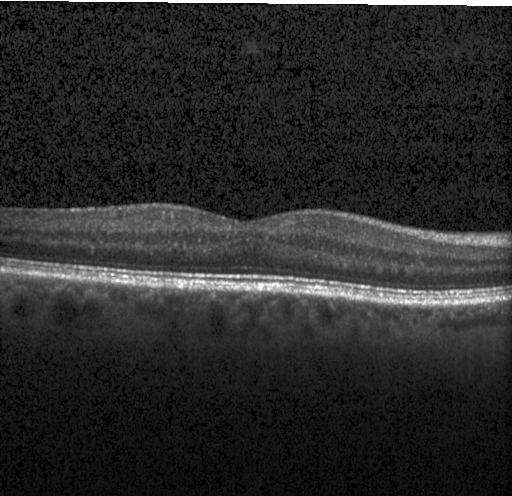

Macular OCT demonstrating no choroidal neovascularization, diabetic macular edema, or drusen.